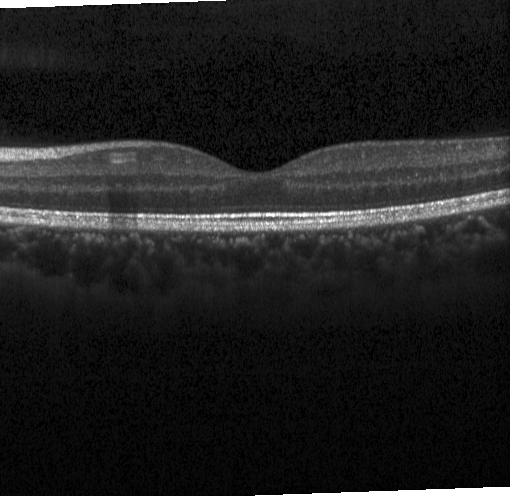
Retinal OCT cross-section · Heidelberg Spectralis. Finding: no choroidal neovascularization, no diabetic macular edema, and no drusen.